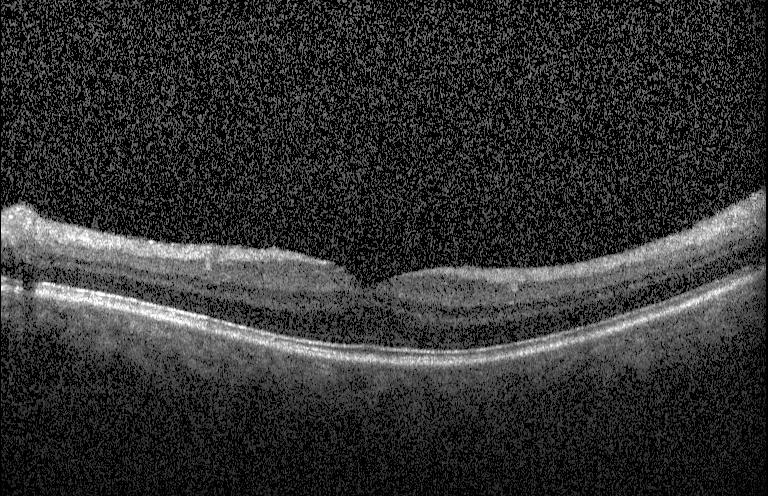
Retinal OCT cross-section showing neither CNV, DME, nor drusen.